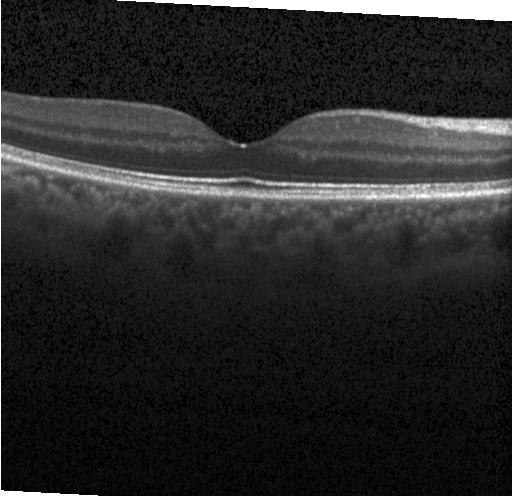
Spectral-domain optical coherence tomography; through the macula; optical coherence tomography B-scan — Diagnosis: no evidence of choroidal neovascularization, diabetic macular edema, or drusen.